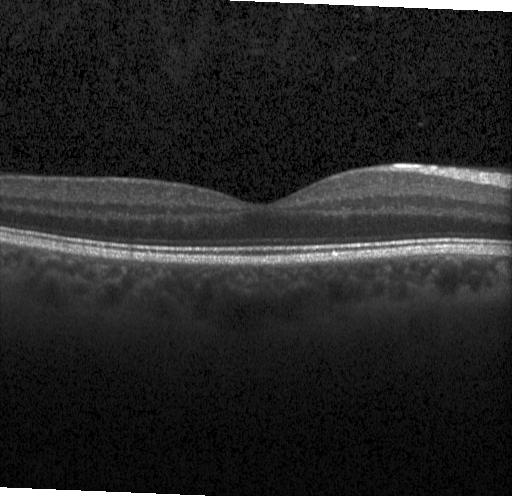

OCT B-scan showing no CNV, no DME, and no drusen.